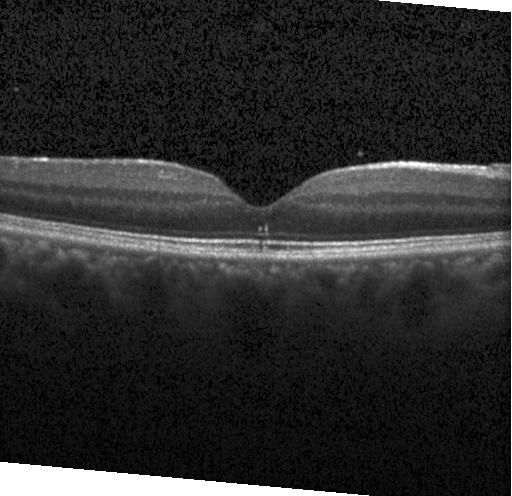

The scan shows no choroidal neovascularization, diabetic macular edema, or drusen.